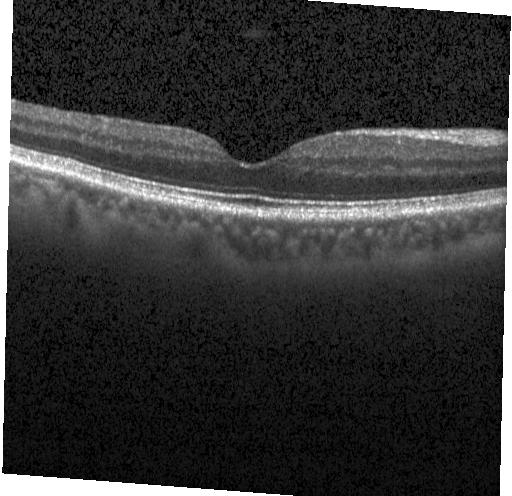 OCT B-scan, instrument: Heidelberg Spectralis, spectral-domain optical coherence tomography, fovea-centered
Diagnosis: no choroidal neovascularization, diabetic macular edema, or drusen.